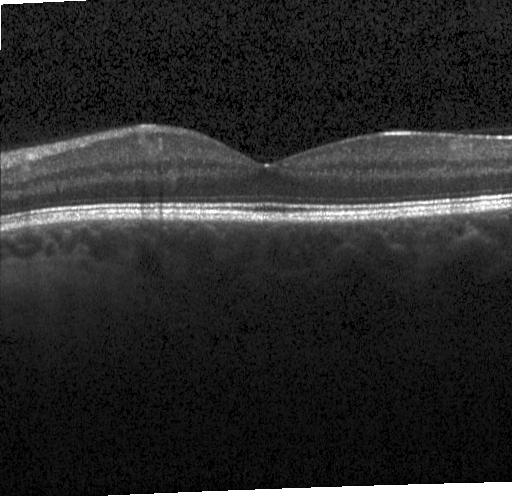
Fovea-centered. Acquired on a Heidelberg Spectralis. Spectral-domain optical coherence tomography. Optical coherence tomography scan — Assessment: neither CNV, DME, nor drusen.